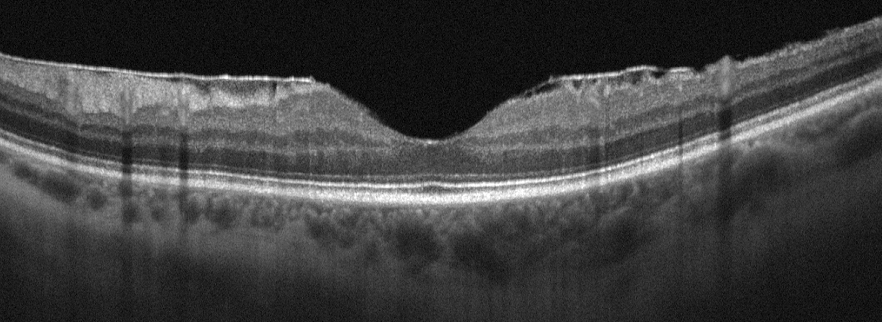

Optical coherence tomography B-scan. Fovea-centered. Optovue Avanti RTVue XR. OS. Macular OCT: epiretinal membrane.